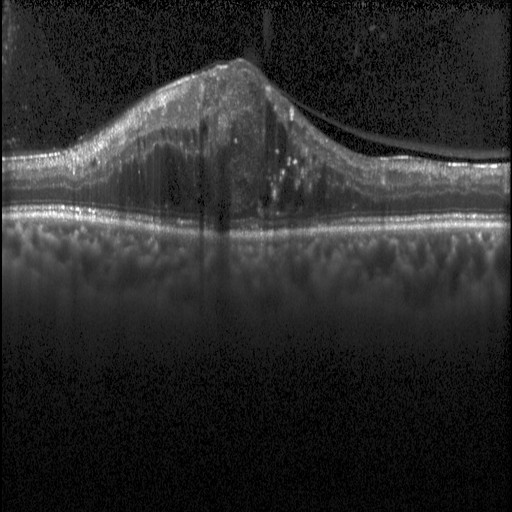 Diagnosis: DME.